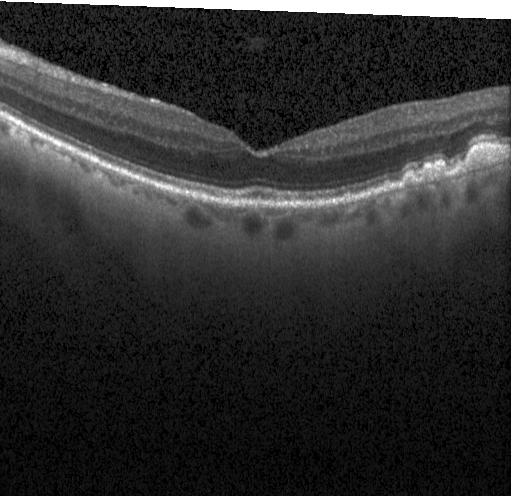 Fovea-centered; instrument: Heidelberg Spectralis; SD-OCT; OCT B-scan — OCT finding: sub-RPE drusenoid deposits.